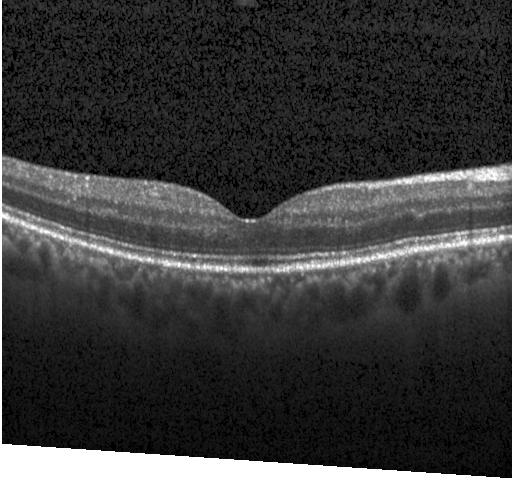
Impression: no evidence of choroidal neovascularization, diabetic macular edema, or drusen.